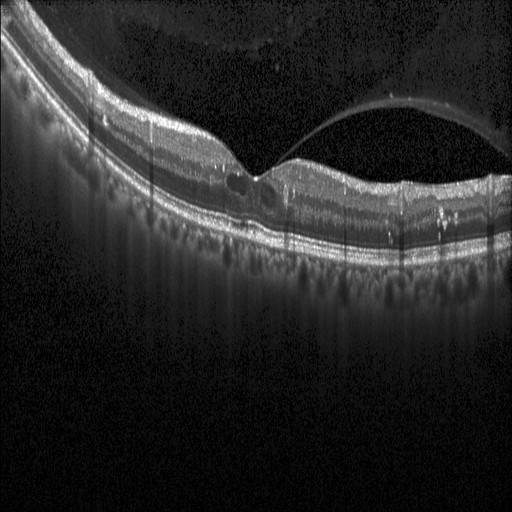
OCT scan showing diabetic macular edema.